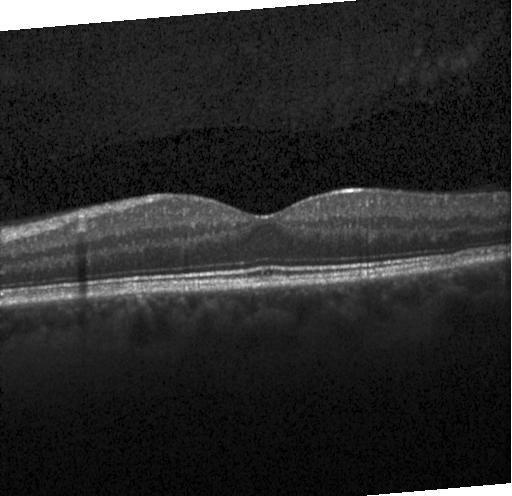

Impression: no evidence of CNV, DME, or drusen.